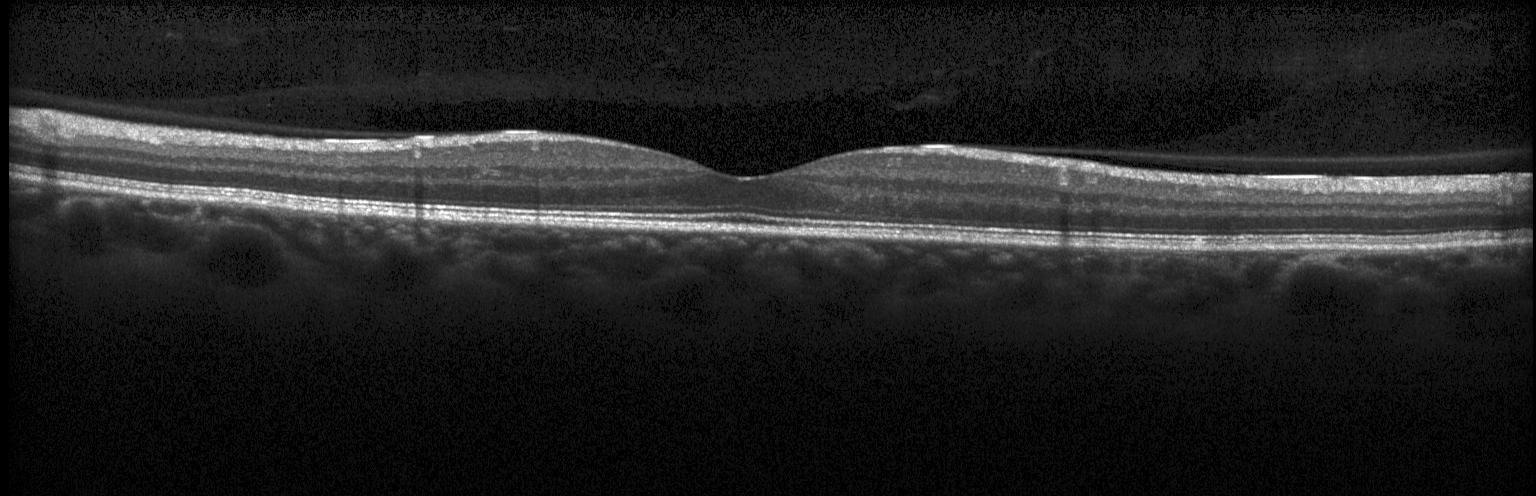
Fovea-centered. Spectral-domain OCT. Heidelberg Spectralis. Retinal OCT B-scan. Impression: neither choroidal neovascularization, diabetic macular edema, nor drusen.